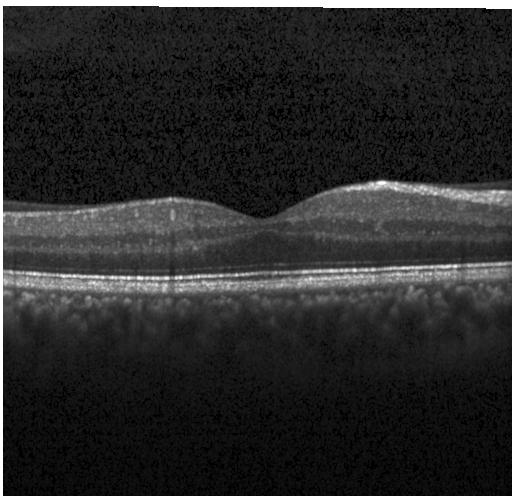

Retinal OCT B-scan · spectral-domain optical coherence tomography · acquired on a Heidelberg Spectralis.
Assessment: no choroidal neovascularization, no diabetic macular edema, and no drusen.